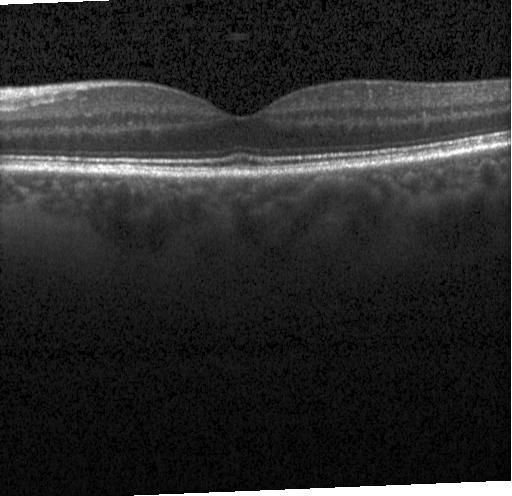 OCT line scan, fovea-centered, SD-OCT.
OCT finding: no evidence of CNV, DME, or drusen.